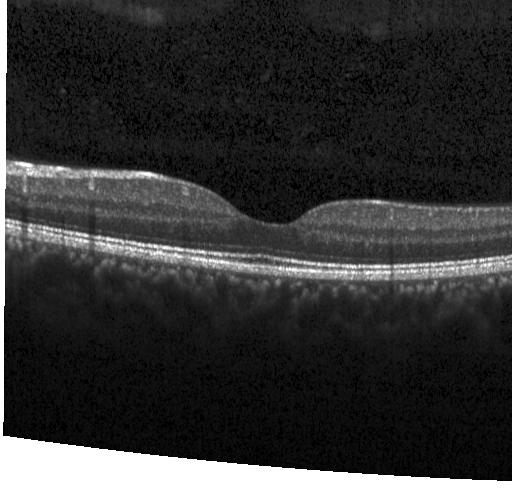

Retinal OCT cross-section. Spectral-domain OCT. Fovea-centered — Dx: no choroidal neovascularization, diabetic macular edema, or drusen.